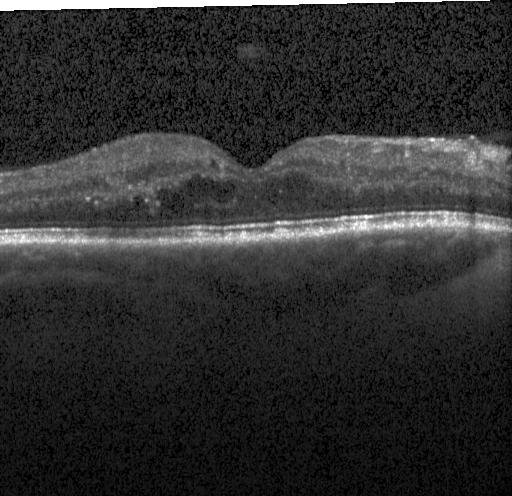 Retinal OCT cross-section. OCT finding: diabetic macular edema.